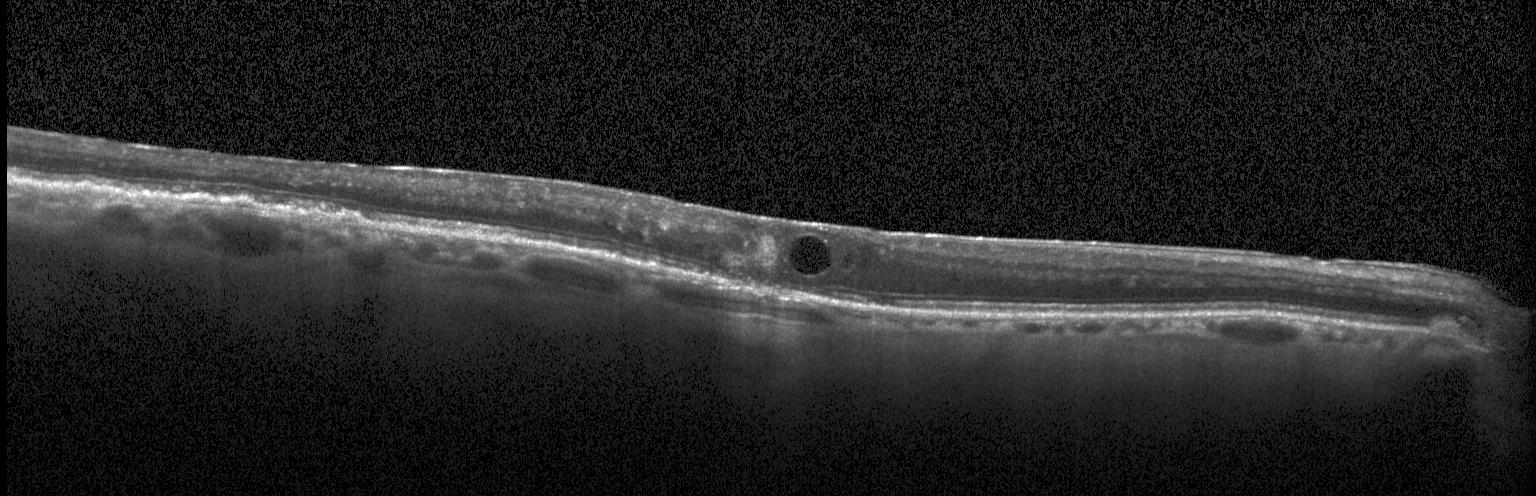 This B-scan demonstrates CNV.